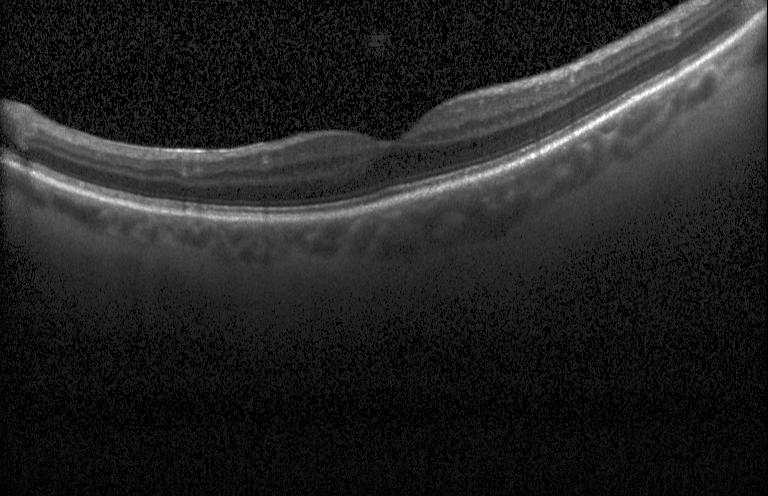

OCT B-scan. Through the macula. Spectral-domain OCT. Heidelberg Spectralis OCT system — Assessment: no choroidal neovascularization, no diabetic macular edema, and no drusen.